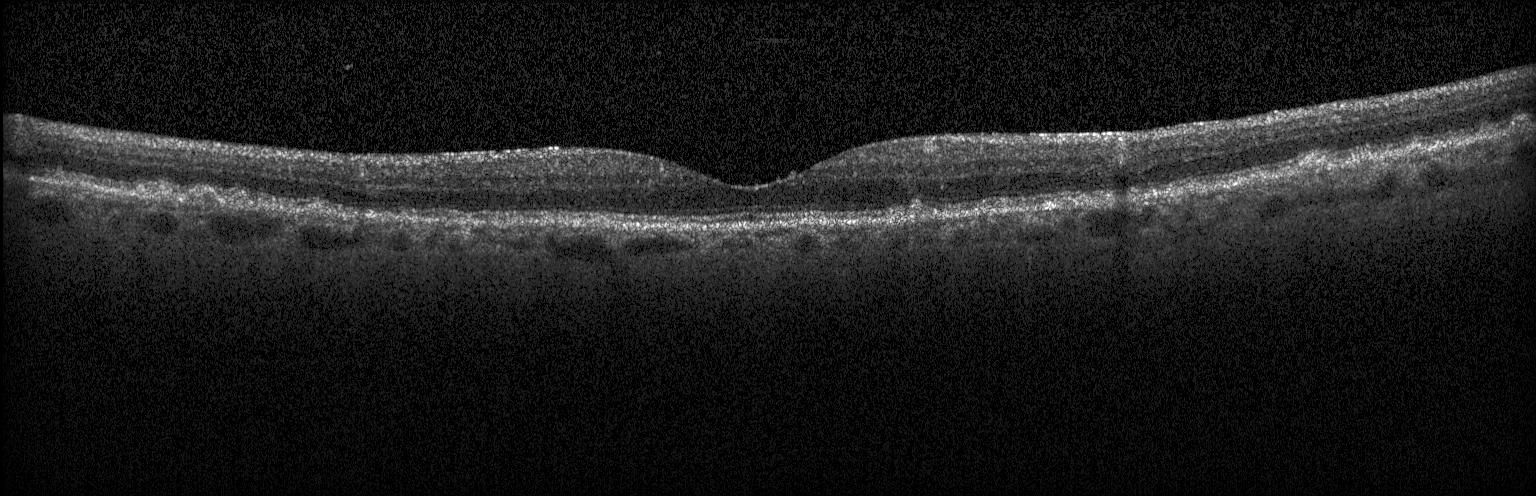 Diagnosis: multiple drusen.